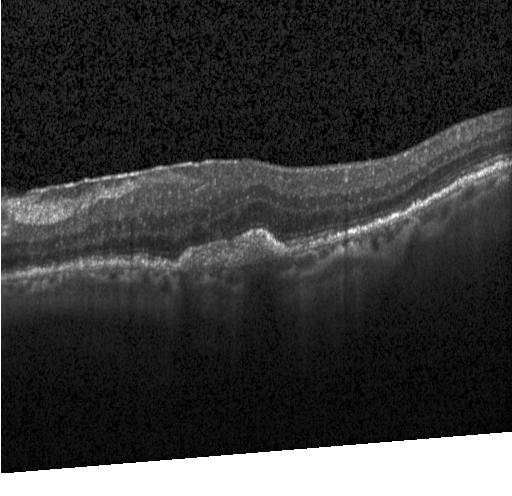

Diagnosis: a choroidal neovascular membrane.